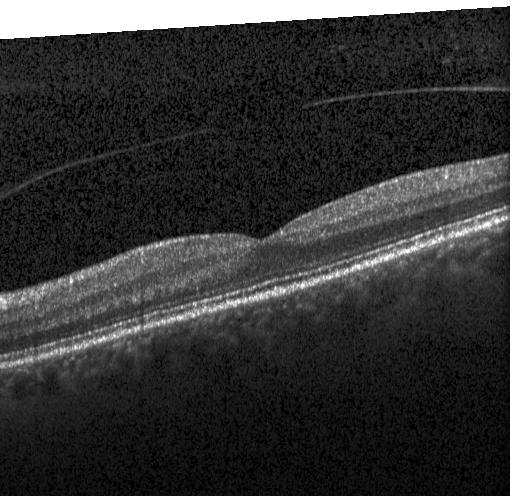

OCT B-scan · centered on the fovea · SD-OCT · instrument: Heidelberg Spectralis.
Impression: no evidence of CNV, DME, or drusen.